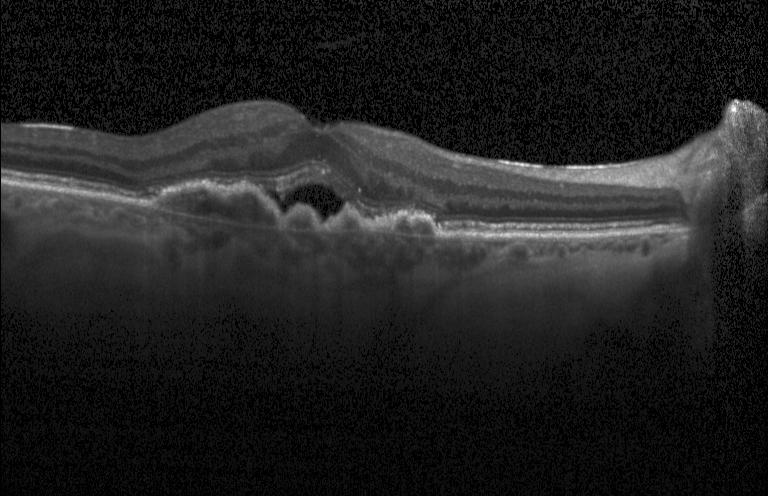
Finding: CNV.